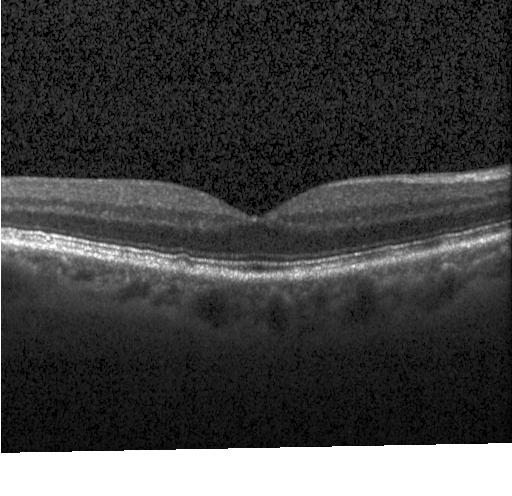
Macular OCT demonstrating sub-RPE drusenoid deposits.